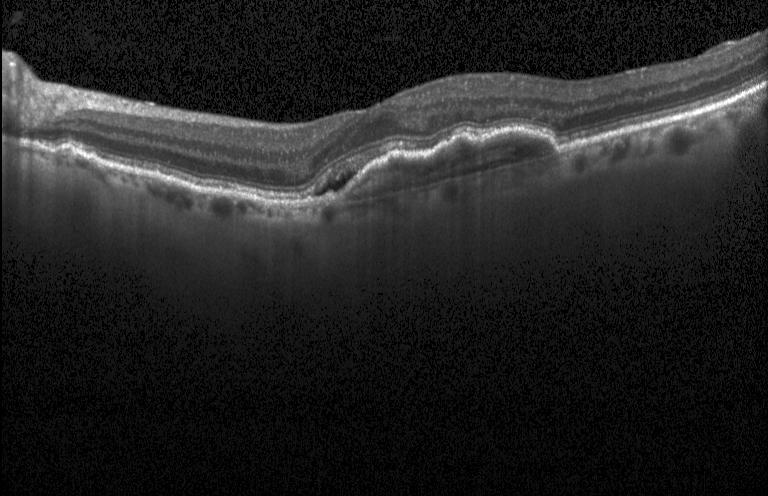

Retinal OCT cross-section. OCT finding: a choroidal neovascular membrane.